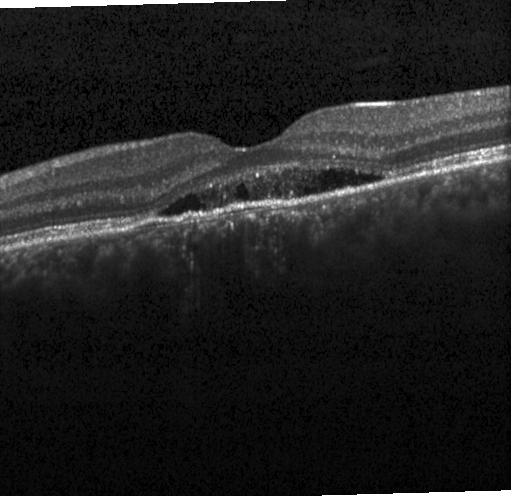 Assessment: a choroidal neovascular membrane.